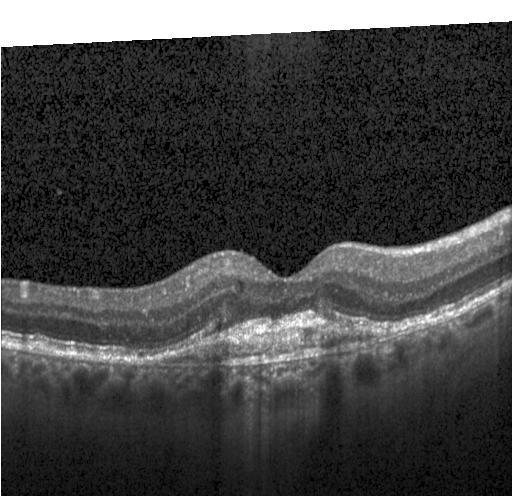
Instrument: Heidelberg Spectralis · OCT B-scan — Dx: choroidal neovascularization.